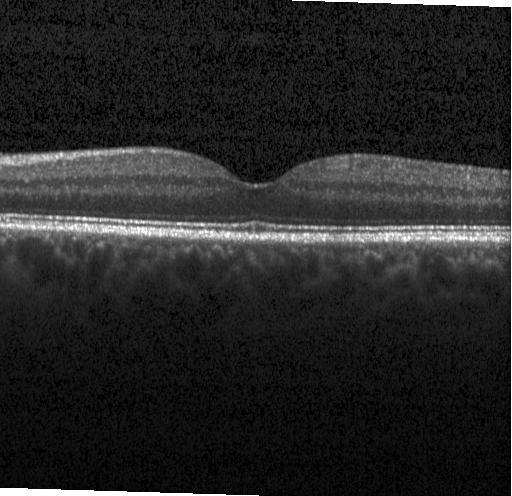 Macular OCT demonstrating no evidence of choroidal neovascularization, diabetic macular edema, or drusen.